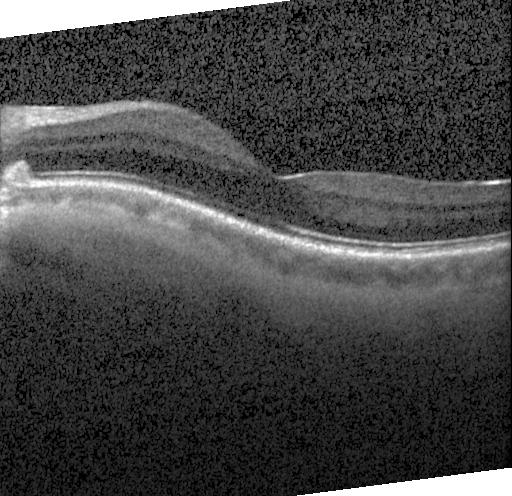

Optical coherence tomography scan. Assessment: drusen.